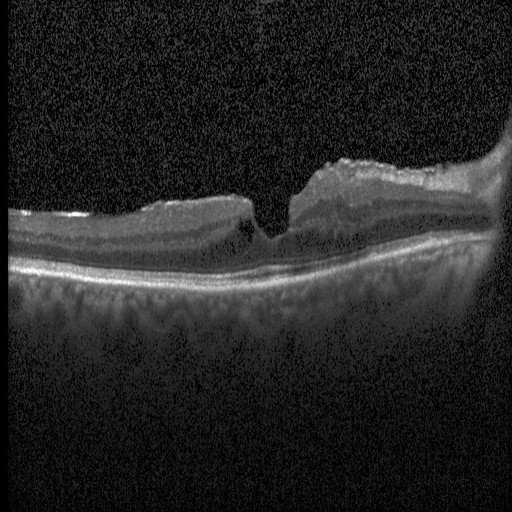 Spectral-domain OCT, acquired on a Heidelberg Spectralis, retinal OCT B-scan, macular scan — This B-scan demonstrates diabetic macular edema (DME).